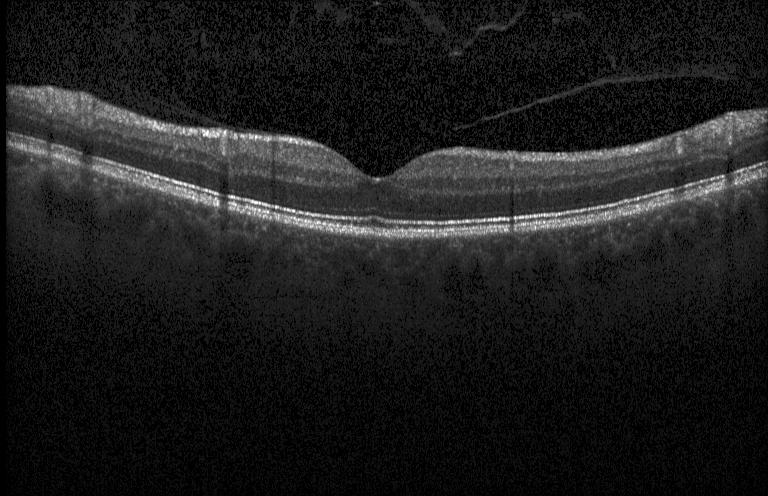
OCT line scan; Heidelberg Spectralis; macular scan; spectral-domain OCT
Macular OCT: no CNV, no DME, and no drusen.